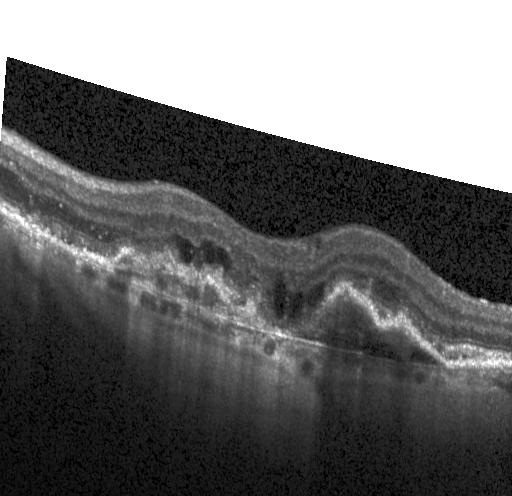

Diagnosis: a choroidal neovascular membrane.